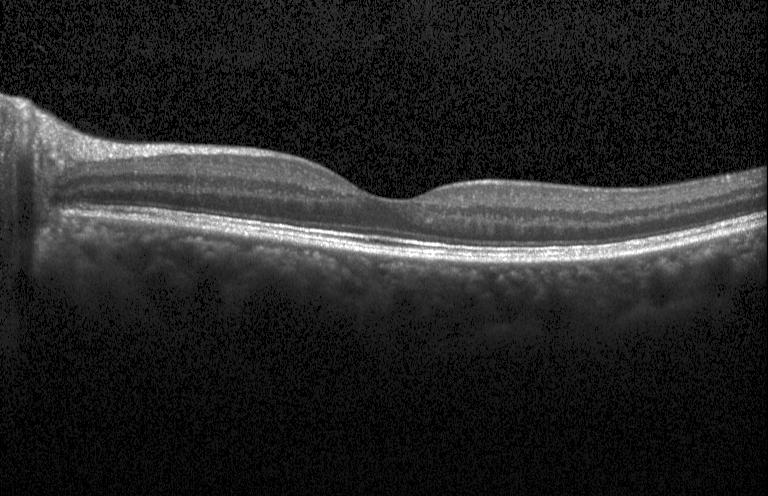

Spectral-domain OCT B-scan: no choroidal neovascularization, no diabetic macular edema, and no drusen.